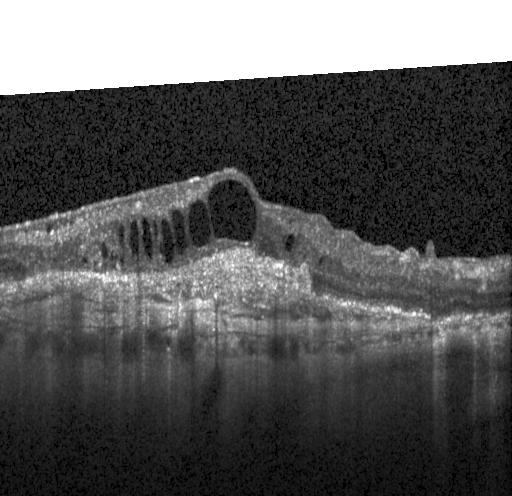 Retinal OCT cross-section showing CNV.